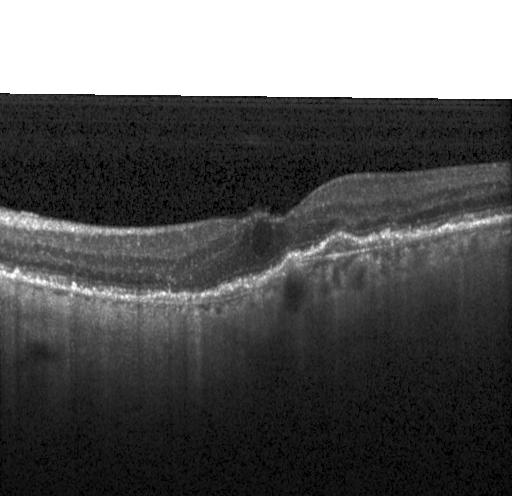
A choroidal neovascular membrane.